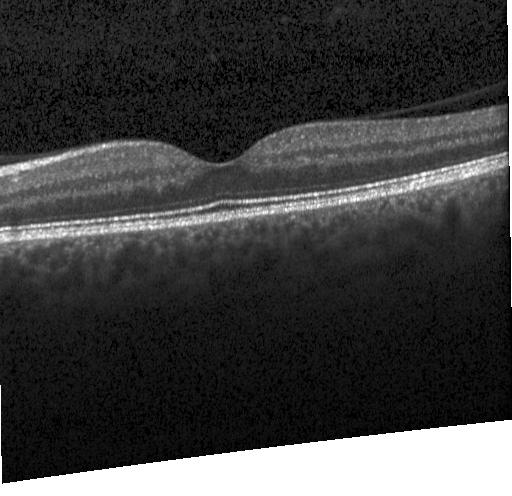
Instrument: Heidelberg Spectralis. Retinal OCT B-scan. Spectral-domain OCT
Diagnosis: no choroidal neovascularization, diabetic macular edema, or drusen.